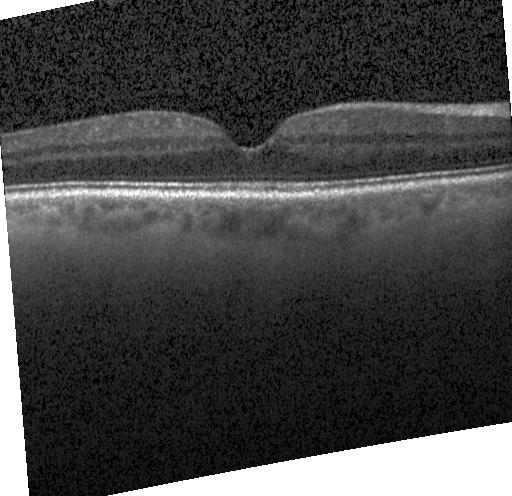
Dx: no CNV, DME, or drusen.